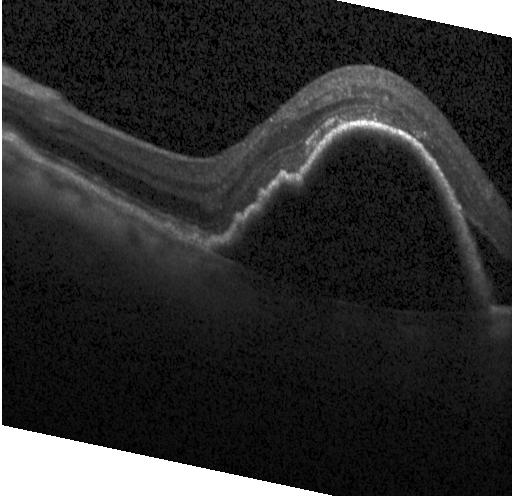
Acquired on a Heidelberg Spectralis; horizontal scan through the fovea; optical coherence tomography B-scan — This B-scan demonstrates a choroidal neovascular membrane.